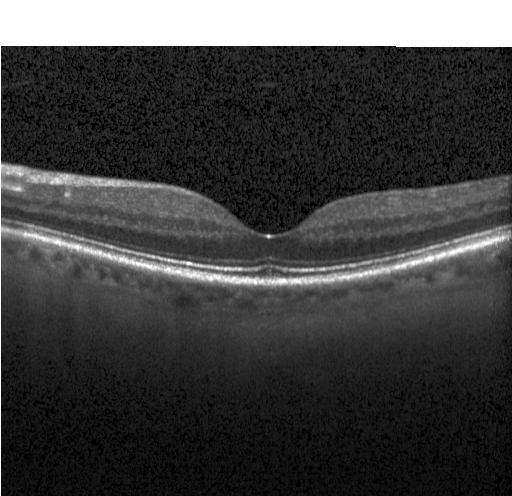
Retinal OCT B-scan
Macular OCT: no evidence of CNV, DME, or drusen.